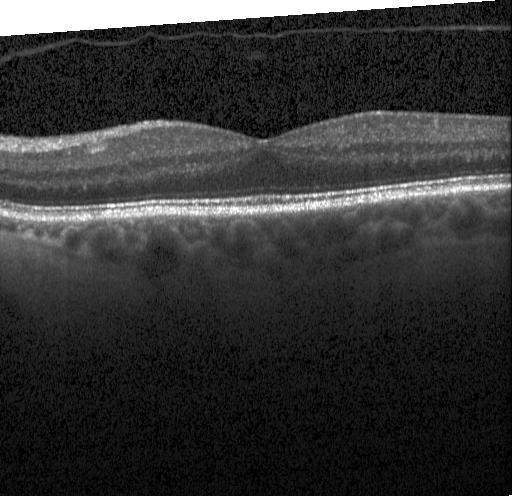 OCT B-scan showing no CNV, DME, or drusen.